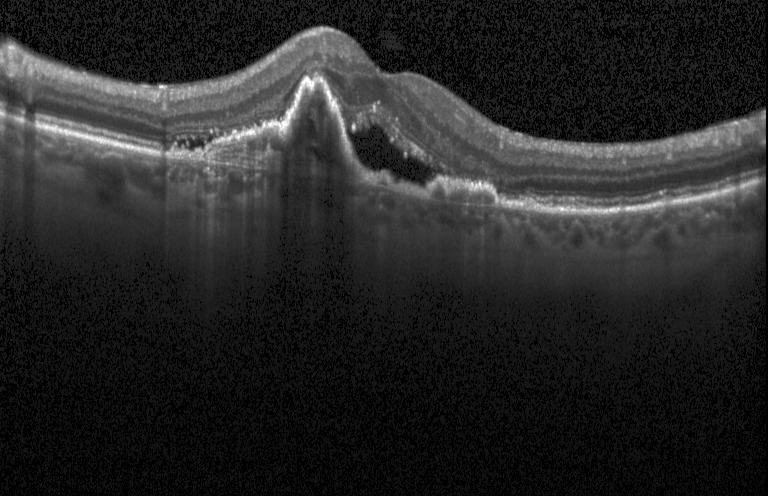 Retinal OCT cross-section showing choroidal neovascularization.